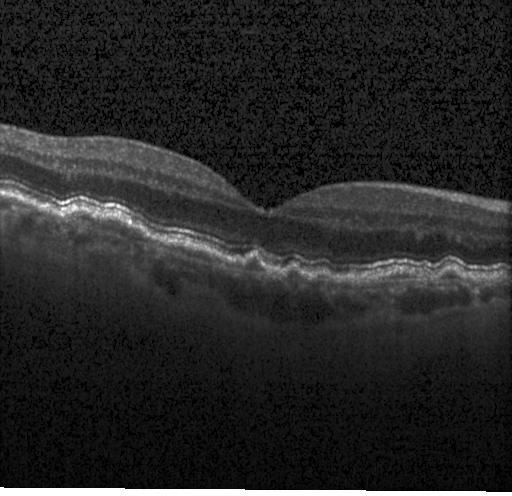
Impression: sub-RPE drusenoid deposits.